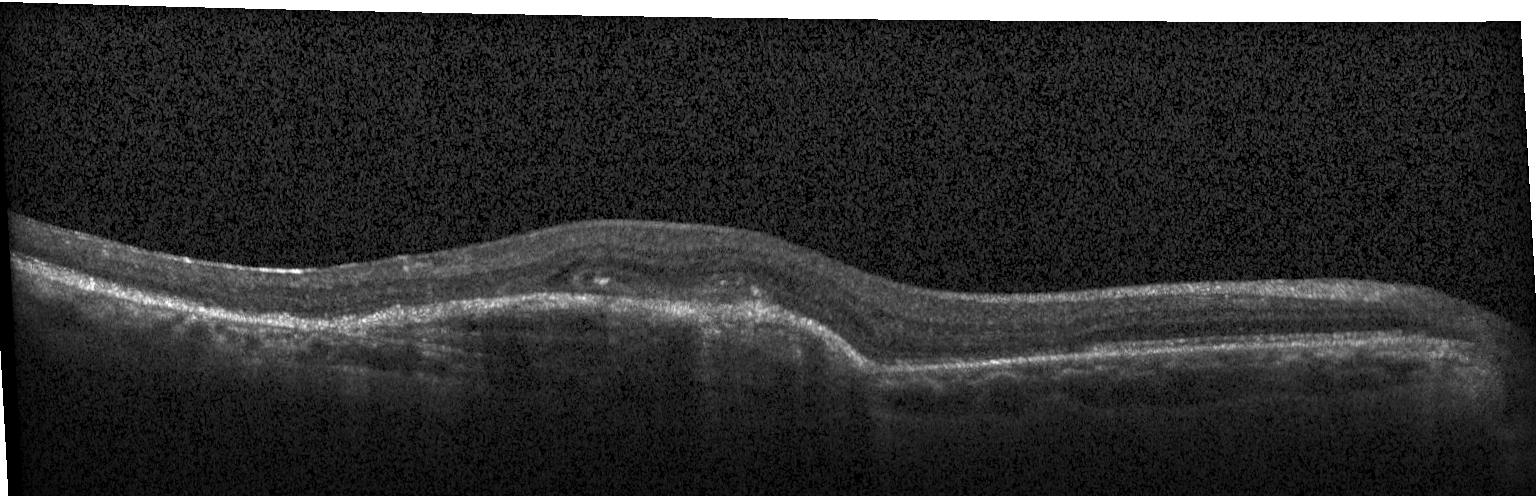 Retinal OCT B-scan. Heidelberg Spectralis. OCT finding: a choroidal neovascular membrane.